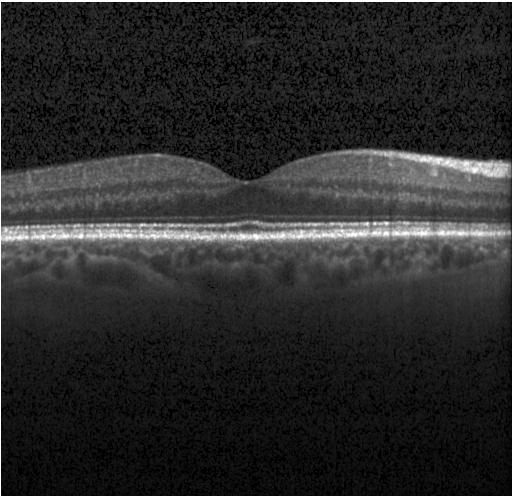

OCT B-scan. SD-OCT. No evidence of CNV, DME, or drusen.